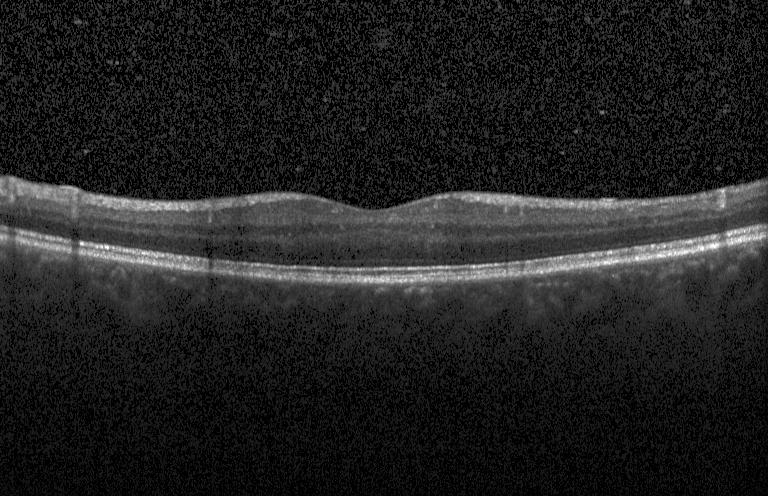
Retinal OCT B-scan
Finding: no evidence of choroidal neovascularization, diabetic macular edema, or drusen.